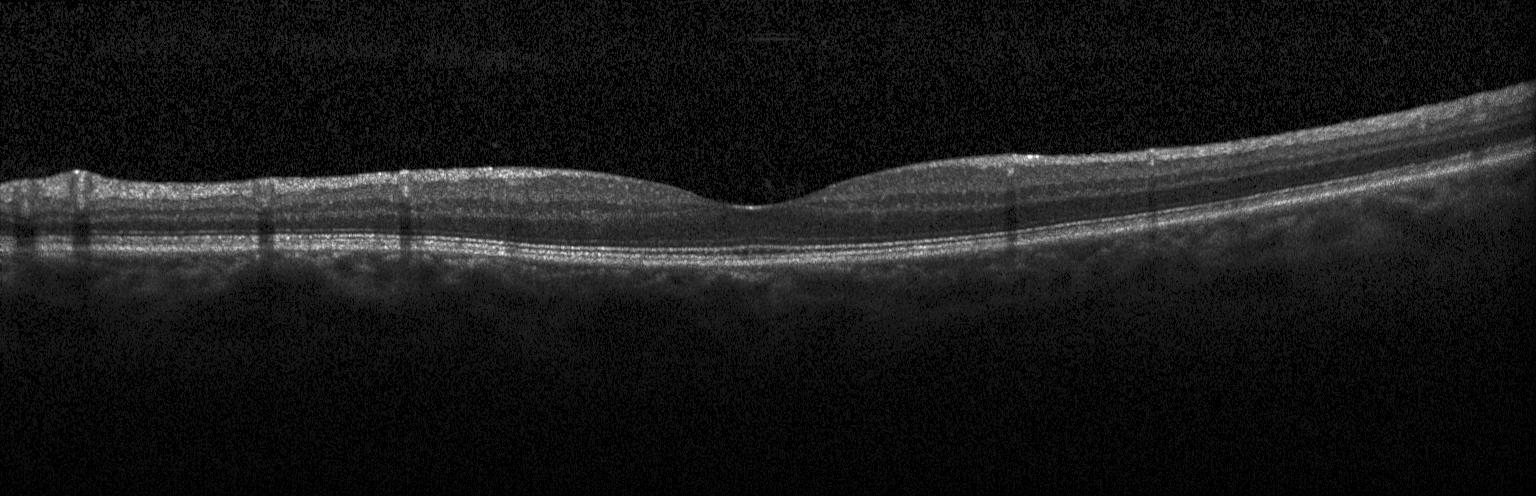
Spectral-domain OCT. Macular scan. Heidelberg Spectralis. OCT line scan.
Diagnosis: no evidence of choroidal neovascularization, diabetic macular edema, or drusen.